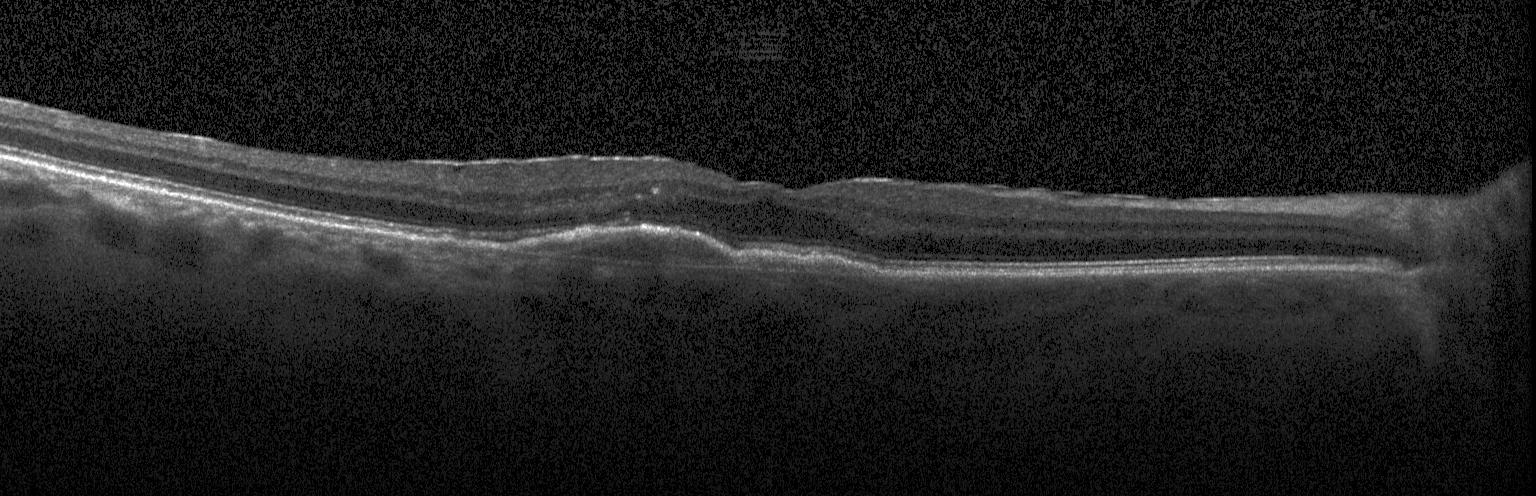
OCT line scan; Heidelberg Spectralis OCT system. Diagnosis: CNV.